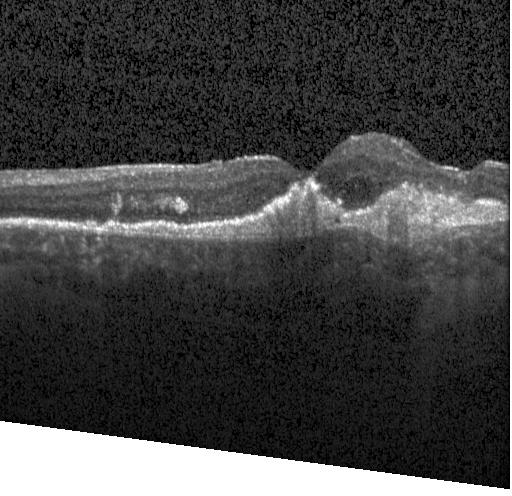
Spectral-domain optical coherence tomography; centered on the fovea; instrument: Heidelberg Spectralis; retinal OCT B-scan — The scan shows choroidal neovascularization (CNV).